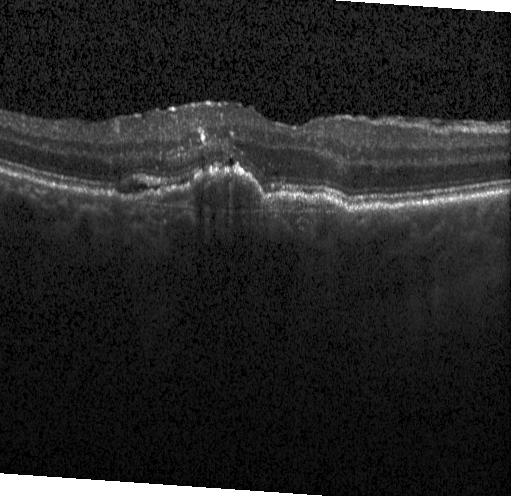

Macular scan. Acquired on a Heidelberg Spectralis. Retinal OCT B-scan.
Diagnosis: choroidal neovascularization.